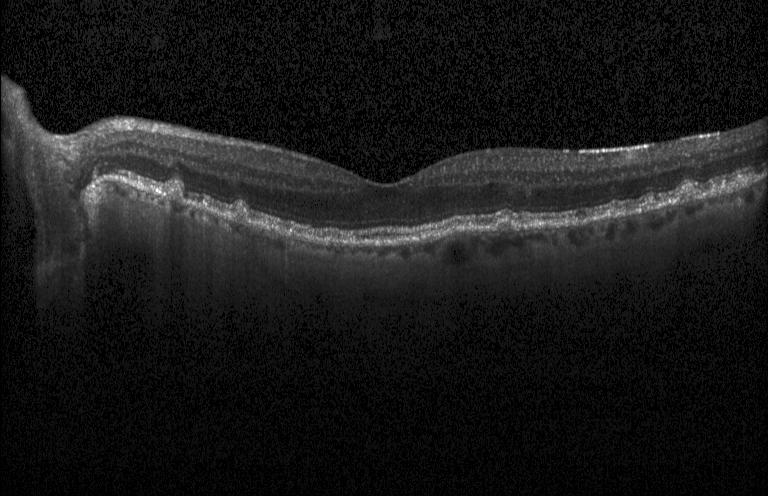

Spectral-domain OCT, optical coherence tomography scan
Drusen.